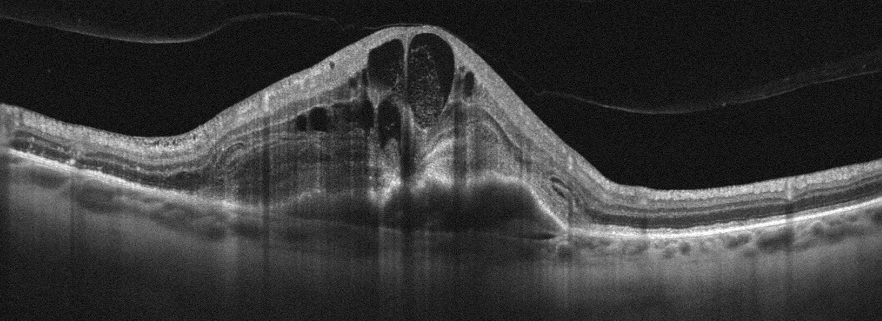
Instrument: Optovue Avanti RTVue XR. OCT B-scan
This B-scan demonstrates age-related macular degeneration (AMD).